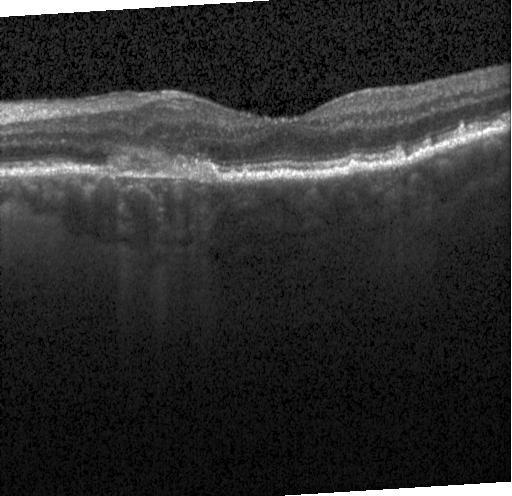
Through the macula; OCT B-scan
OCT finding: choroidal neovascularization (CNV).